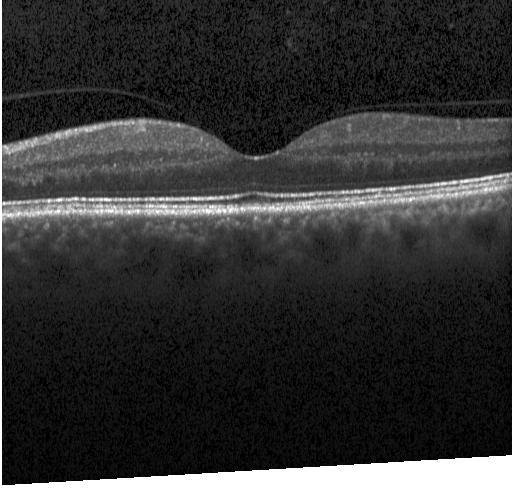
Macular OCT: neither choroidal neovascularization, diabetic macular edema, nor drusen.